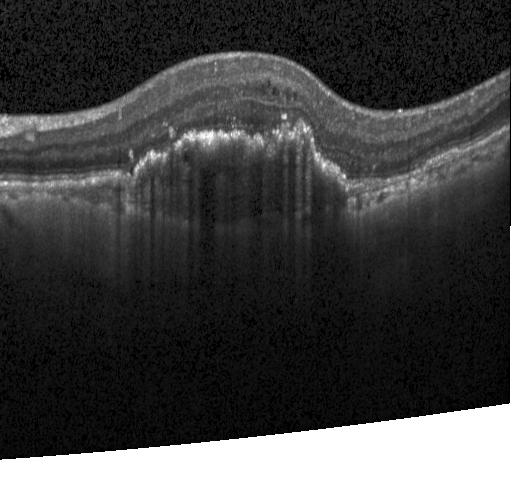 Finding: a choroidal neovascular membrane.